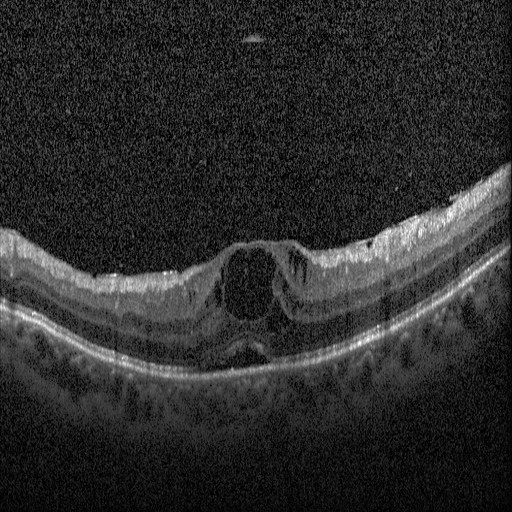
Retinal OCT B-scan. Diabetic macular edema (DME).